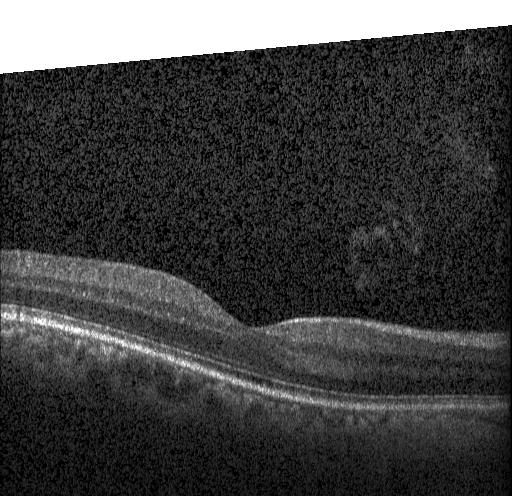

OCT B-scan; fovea-centered; Heidelberg Spectralis OCT system; spectral-domain OCT.
Impression: no CNV, no DME, and no drusen.